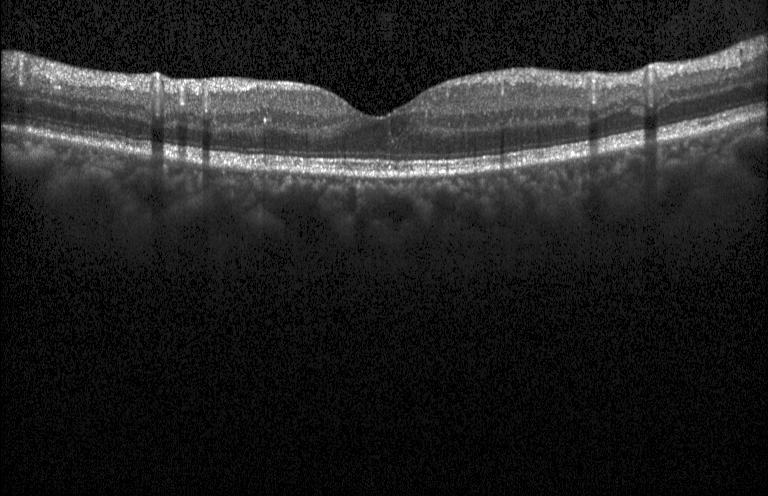 Instrument: Heidelberg Spectralis. Optical coherence tomography scan. SD-OCT. Centered on the fovea.
Dx: no choroidal neovascularization, no diabetic macular edema, and no drusen.